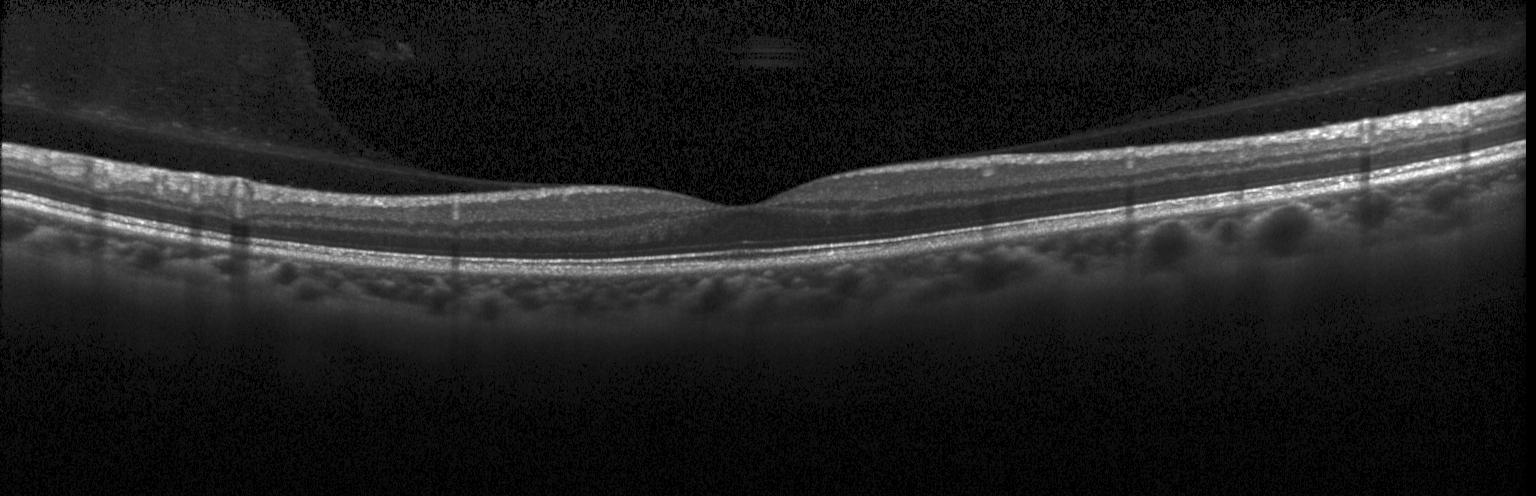
Through the macula · retinal OCT cross-section · Heidelberg Spectralis. Diagnosis: no evidence of choroidal neovascularization, diabetic macular edema, or drusen.